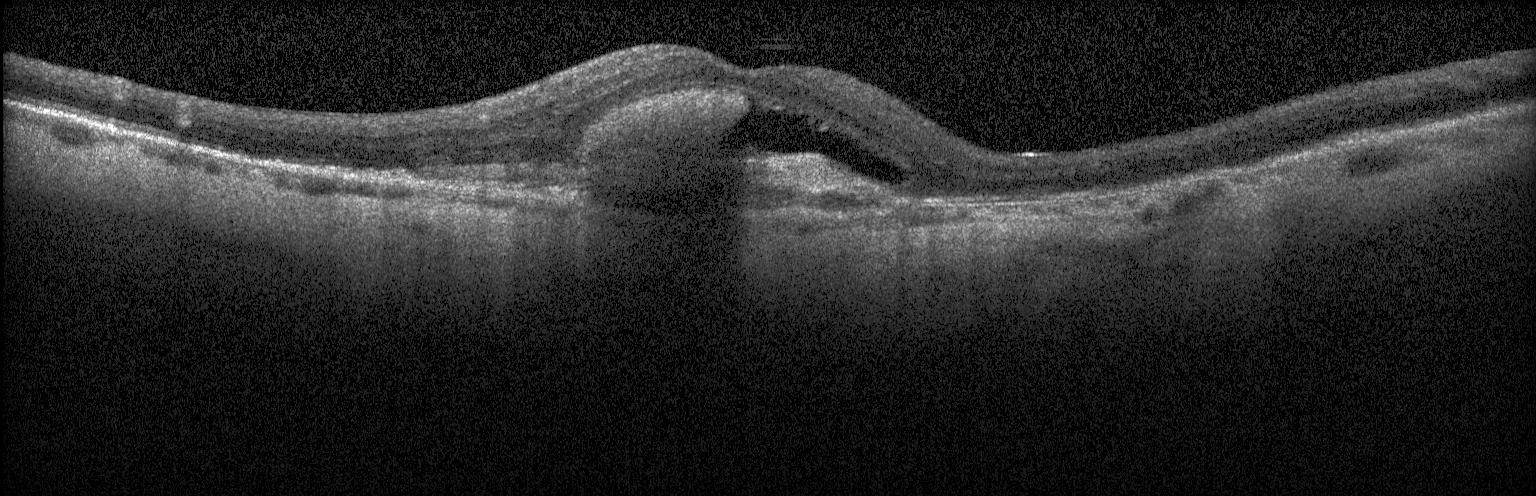
Heidelberg Spectralis OCT system, OCT line scan, spectral-domain optical coherence tomography, centered on the fovea.
Finding: choroidal neovascularization.